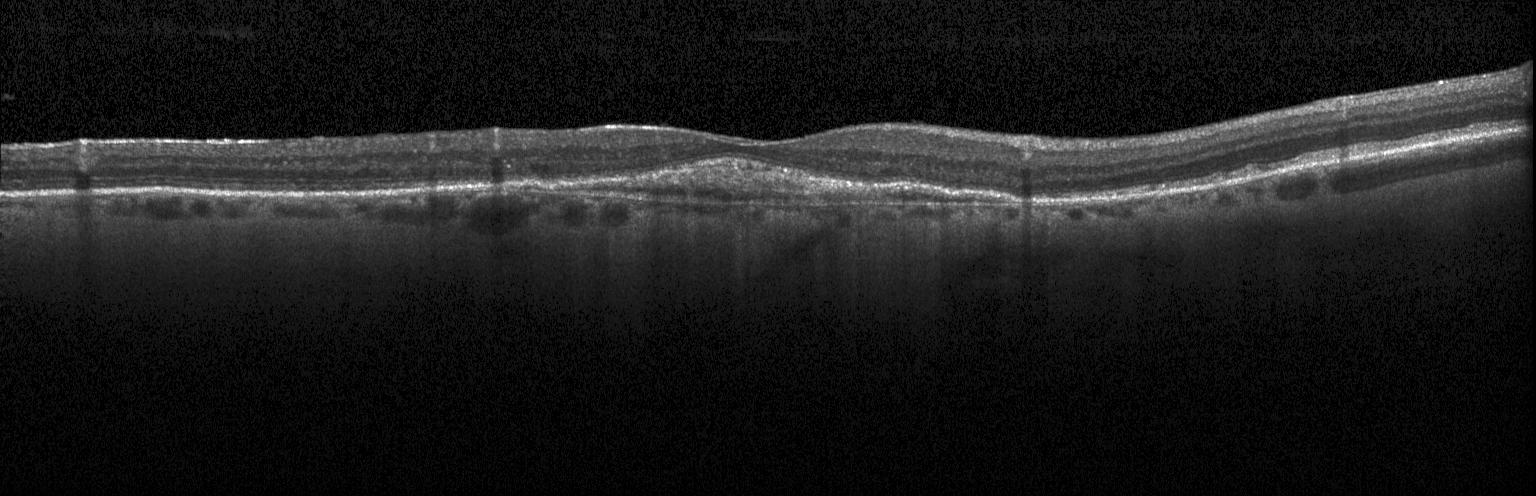

Optical coherence tomography scan; acquired on a Heidelberg Spectralis; through the macula; SD-OCT.
Impression: a choroidal neovascular membrane.